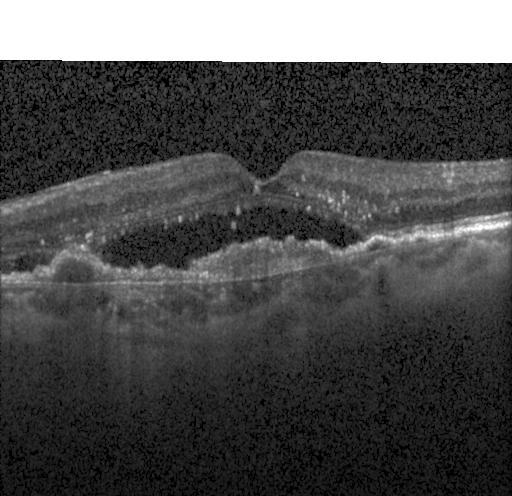

SD-OCT, Heidelberg Spectralis OCT system, retinal OCT cross-section — Dx: a choroidal neovascular membrane.